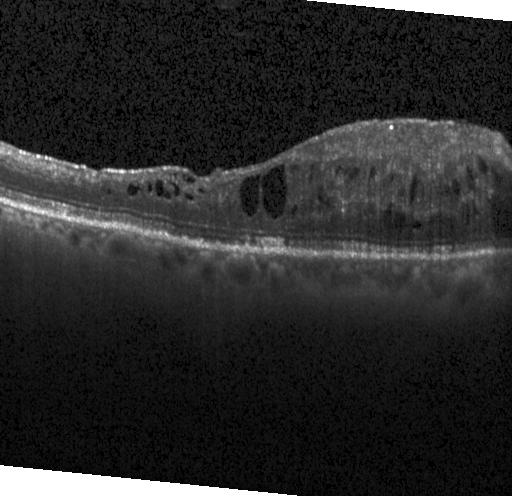

Macular scan; optical coherence tomography B-scan. Diagnosis: DME.